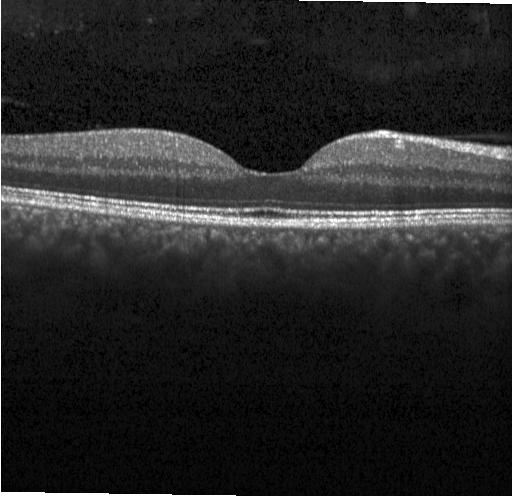
Retinal OCT B-scan. Through the macula. Diagnosis: no evidence of choroidal neovascularization, diabetic macular edema, or drusen.